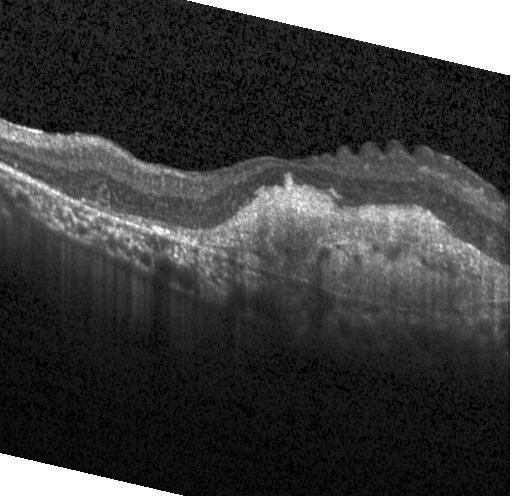 Spectral-domain optical coherence tomography, optical coherence tomography scan, Heidelberg Spectralis OCT system
Finding: a choroidal neovascular membrane.